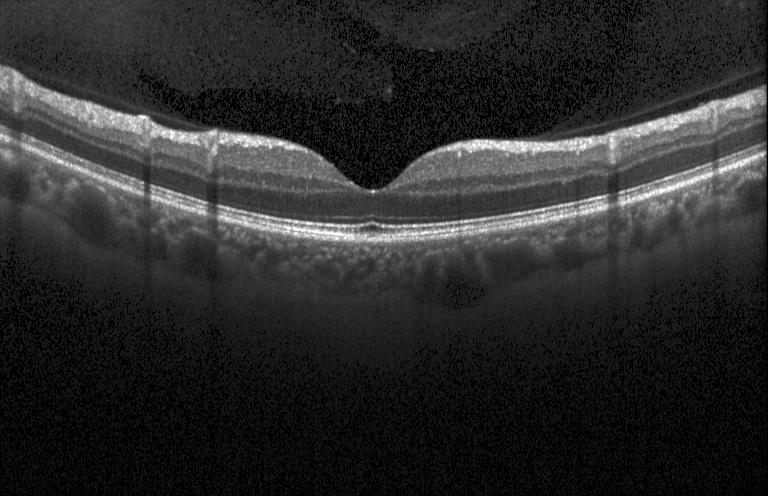
Spectral-domain OCT; OCT line scan.
Finding: no evidence of choroidal neovascularization, diabetic macular edema, or drusen.